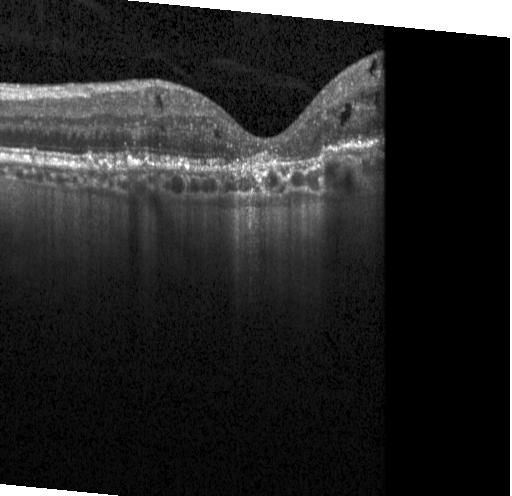
OCT line scan.
Finding: CNV.